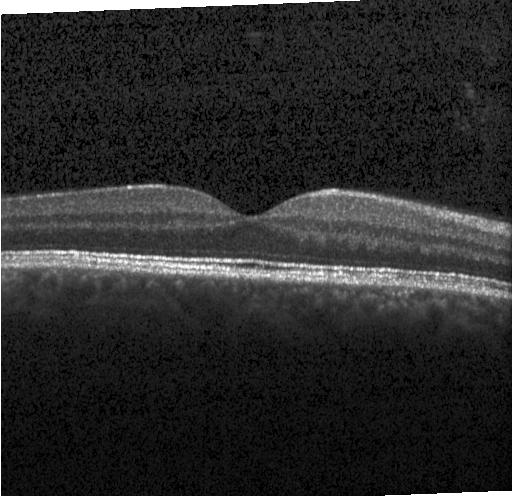 OCT scan showing neither CNV, DME, nor drusen.